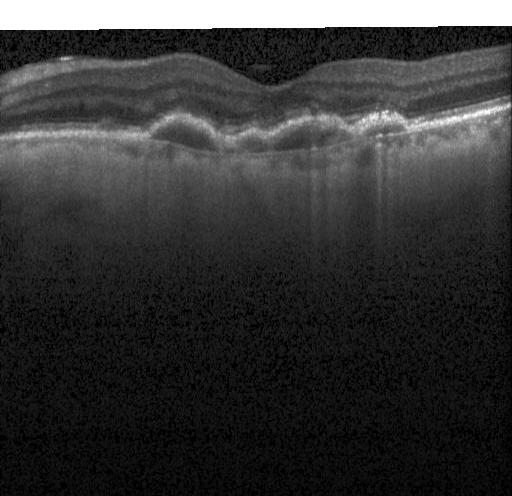

SD-OCT · retinal OCT B-scan — The scan shows a choroidal neovascular membrane.